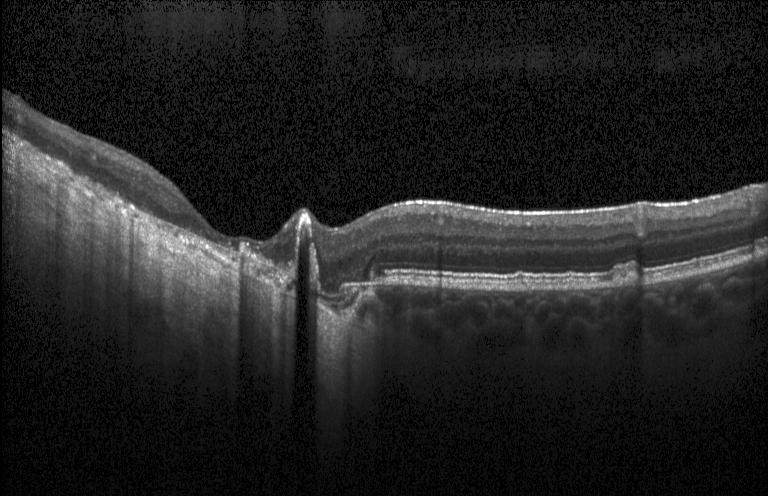

Diagnosis: CNV.